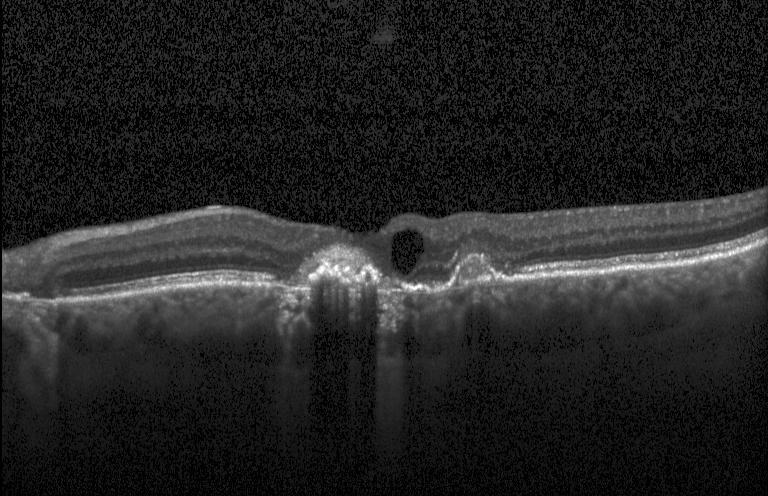 Spectral-domain OCT B-scan: a choroidal neovascular membrane.